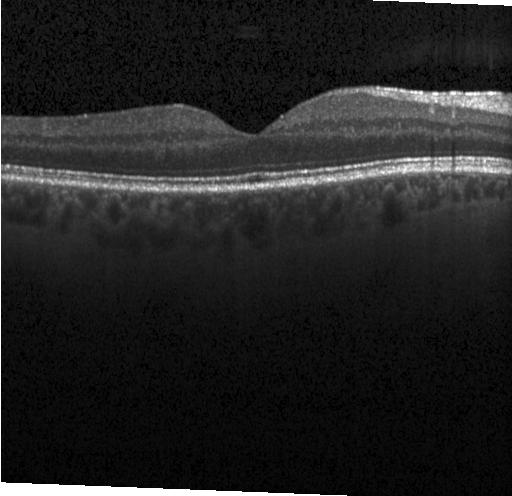 OCT scan showing no choroidal neovascularization, no diabetic macular edema, and no drusen.